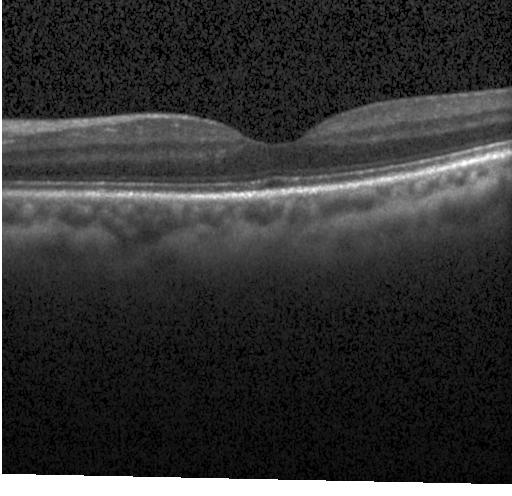 Optical coherence tomography scan, instrument: Heidelberg Spectralis, centered on the fovea. This B-scan demonstrates no evidence of choroidal neovascularization, diabetic macular edema, or drusen.